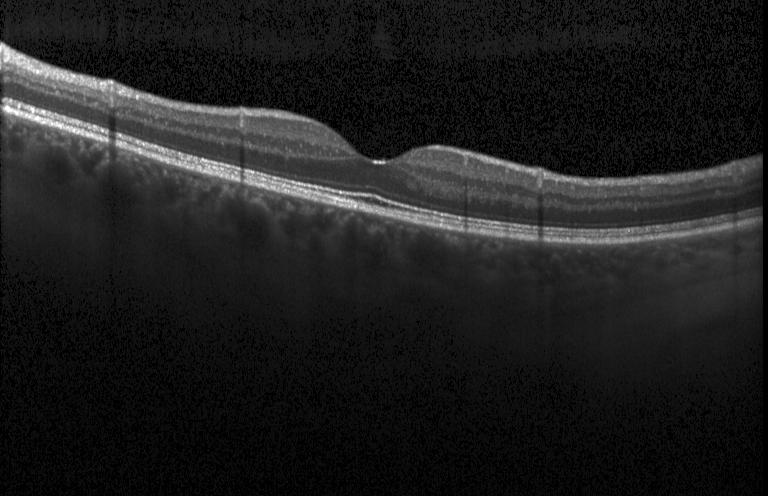
OCT line scan. Impression: neither choroidal neovascularization, diabetic macular edema, nor drusen.